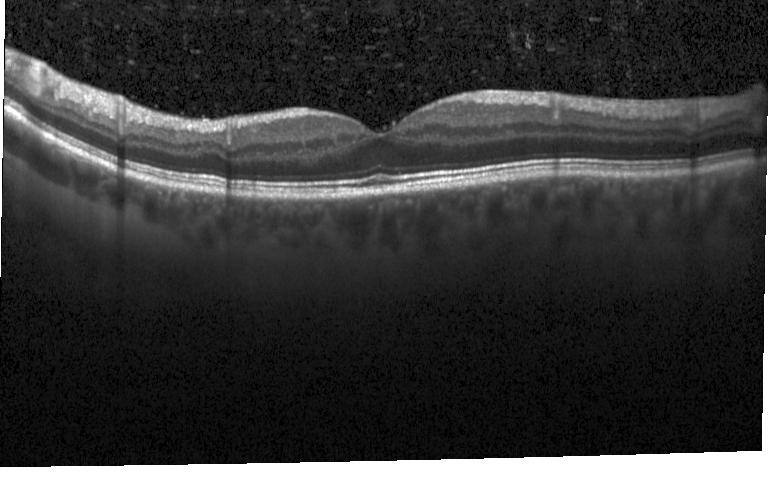

Macular OCT demonstrating neither choroidal neovascularization, diabetic macular edema, nor drusen.